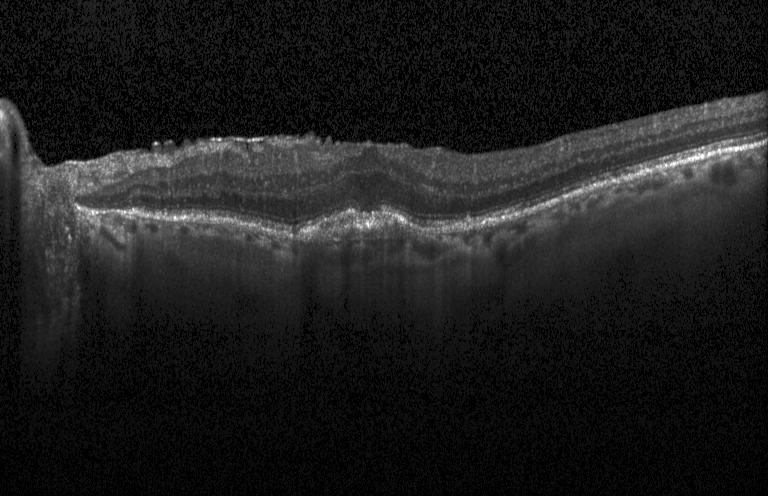
Optical coherence tomography scan, acquired on a Heidelberg Spectralis — Dx: choroidal neovascularization (CNV).